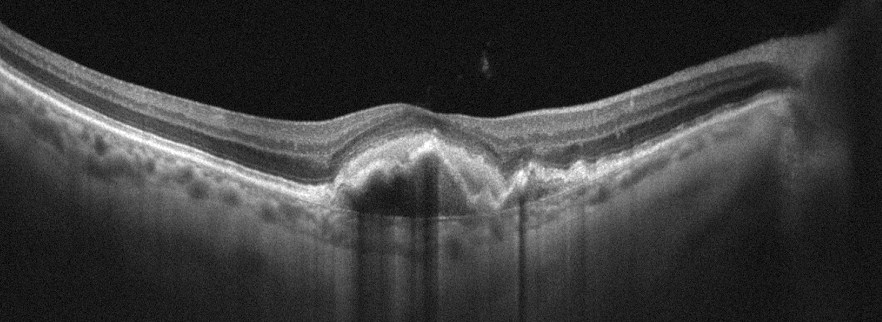

Retinal OCT cross-section
Impression: AMD.